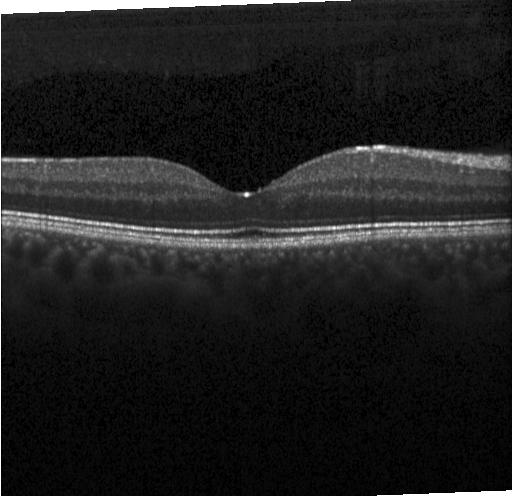 Through the macula · optical coherence tomography scan
Neither choroidal neovascularization, diabetic macular edema, nor drusen.